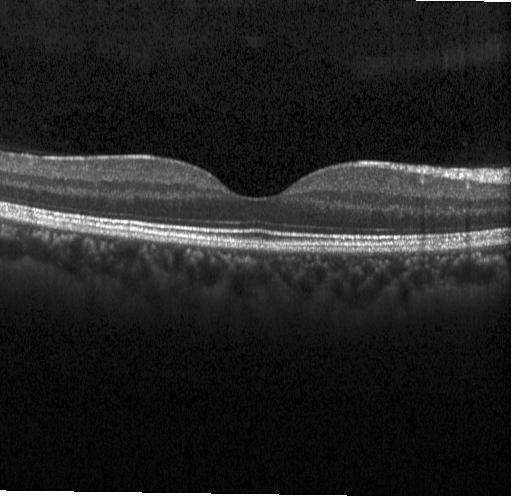 OCT finding: no evidence of choroidal neovascularization, diabetic macular edema, or drusen.